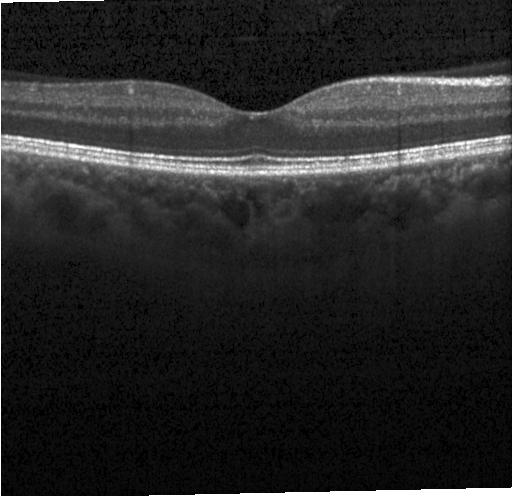 Spectral-domain optical coherence tomography; OCT line scan — This B-scan demonstrates no choroidal neovascularization, diabetic macular edema, or drusen.